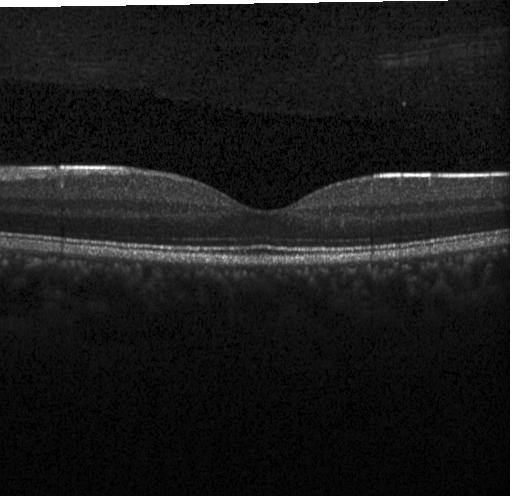 Spectral-domain OCT B-scan: no evidence of CNV, DME, or drusen.